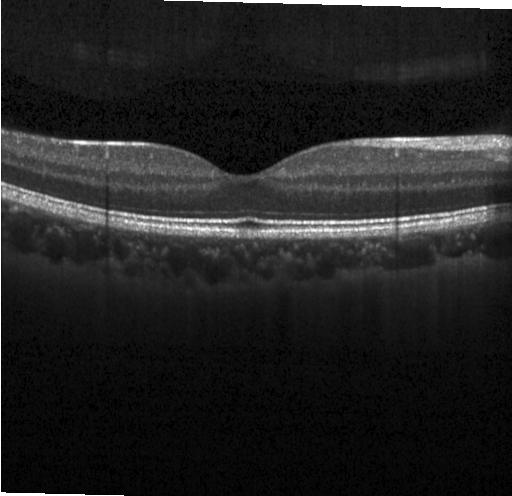
OCT scan showing no CNV, no DME, and no drusen.